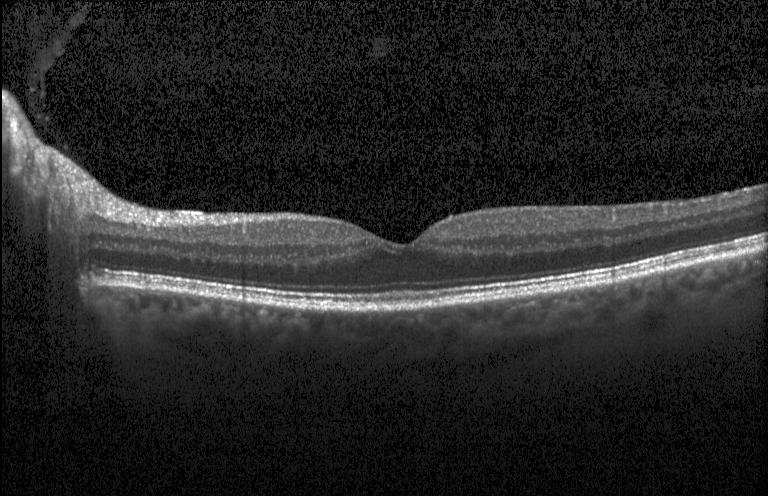
Spectral-domain optical coherence tomography · instrument: Heidelberg Spectralis · fovea-centered · OCT B-scan. Macular OCT: no choroidal neovascularization, diabetic macular edema, or drusen.